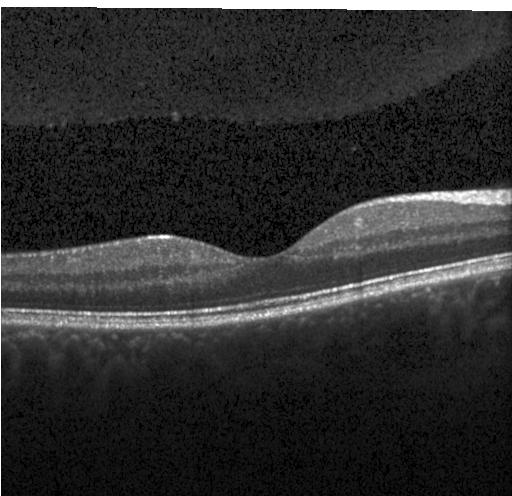

Retinal OCT B-scan · instrument: Heidelberg Spectralis
Diagnosis: neither choroidal neovascularization, diabetic macular edema, nor drusen.